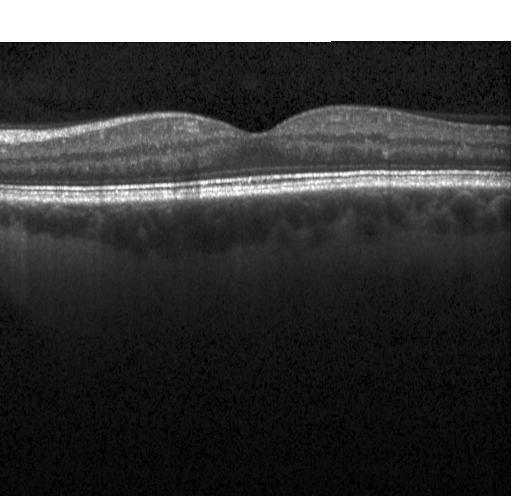
Spectral-domain optical coherence tomography; retinal OCT B-scan
Finding: no evidence of choroidal neovascularization, diabetic macular edema, or drusen.